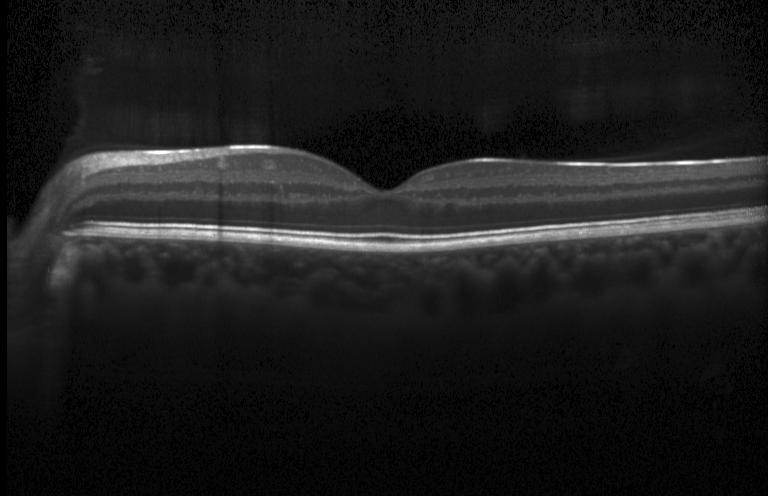 Fovea-centered · OCT line scan. Impression: no choroidal neovascularization, no diabetic macular edema, and no drusen.